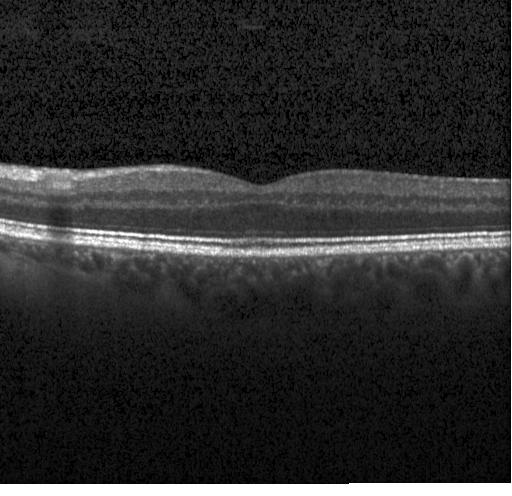
Instrument: Heidelberg Spectralis · OCT B-scan. No evidence of choroidal neovascularization, diabetic macular edema, or drusen.